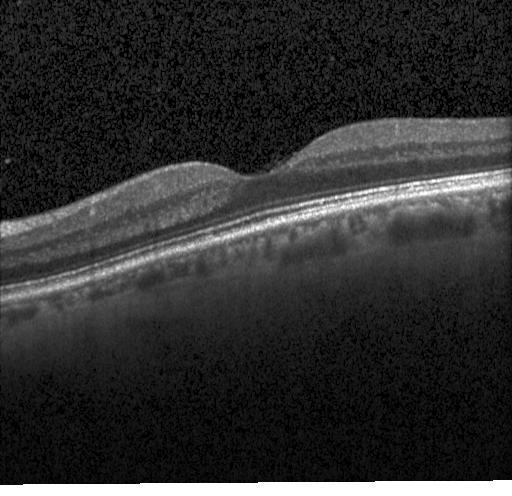 Optical coherence tomography B-scan; through the macula; Heidelberg Spectralis OCT system.
Dx: neither CNV, DME, nor drusen.